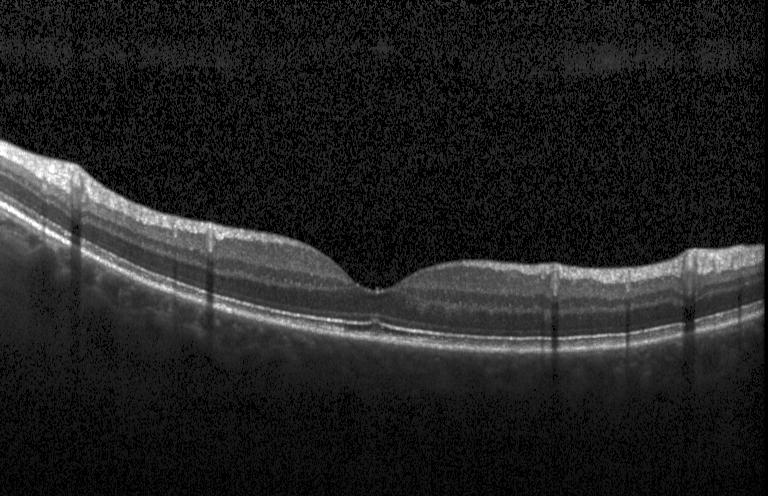 Retinal OCT cross-section · instrument: Heidelberg Spectralis · macular scan. This B-scan demonstrates no CNV, no DME, and no drusen.